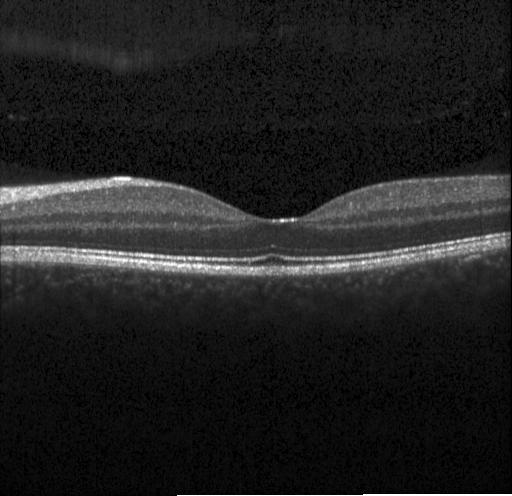
Optical coherence tomography scan.
Impression: no choroidal neovascularization, diabetic macular edema, or drusen.